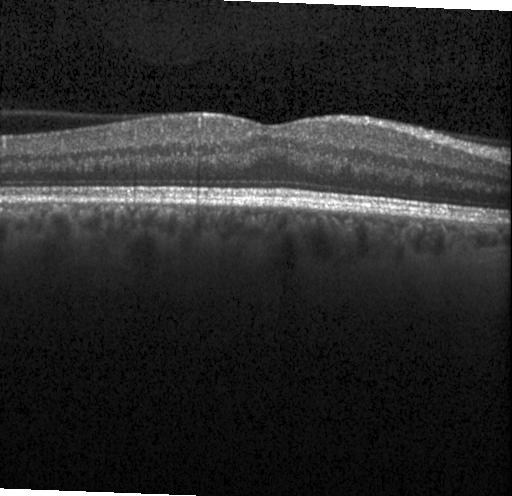
OCT line scan. This B-scan demonstrates no choroidal neovascularization, no diabetic macular edema, and no drusen.